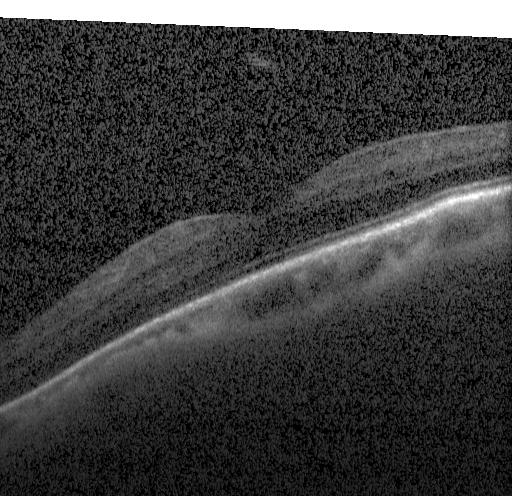 Retinal OCT B-scan — Finding: no choroidal neovascularization, diabetic macular edema, or drusen.